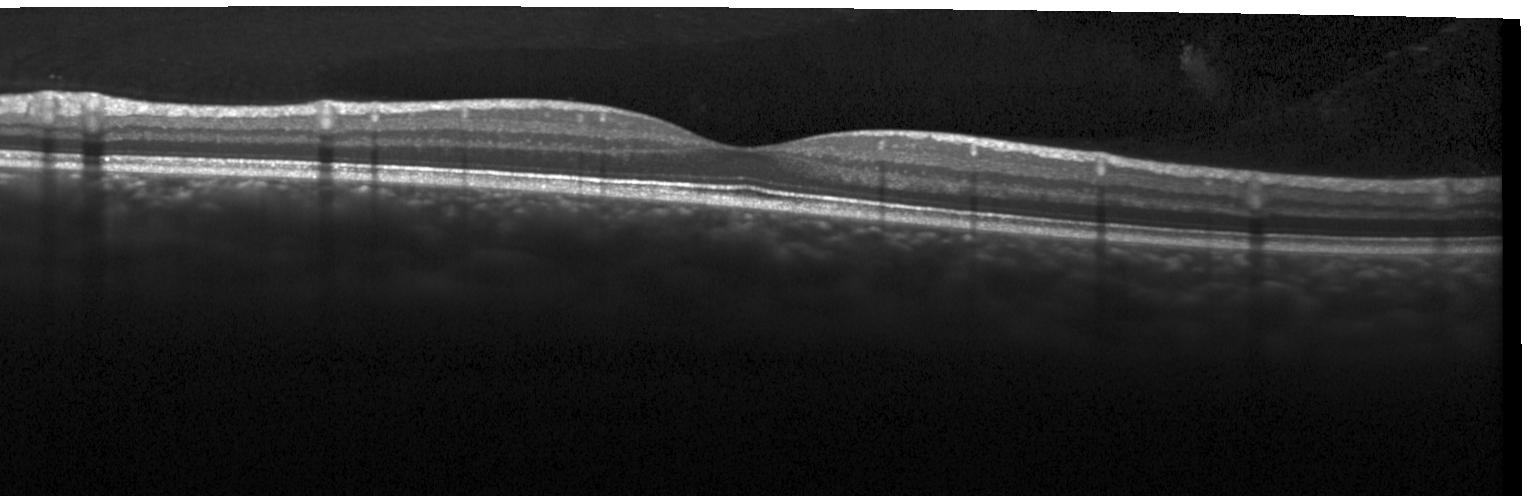
Retinal OCT B-scan. This B-scan demonstrates neither choroidal neovascularization, diabetic macular edema, nor drusen.